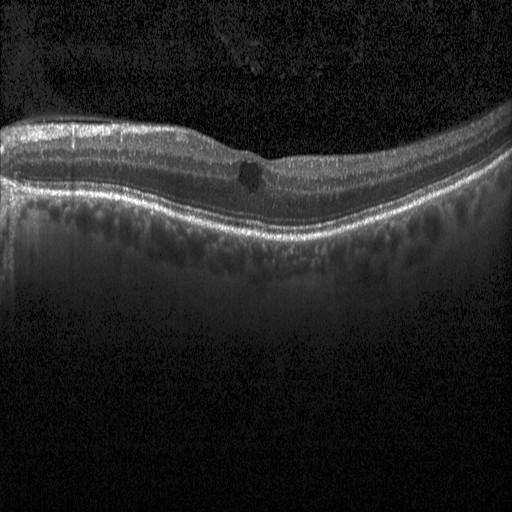 OCT finding: diabetic macular edema (DME).